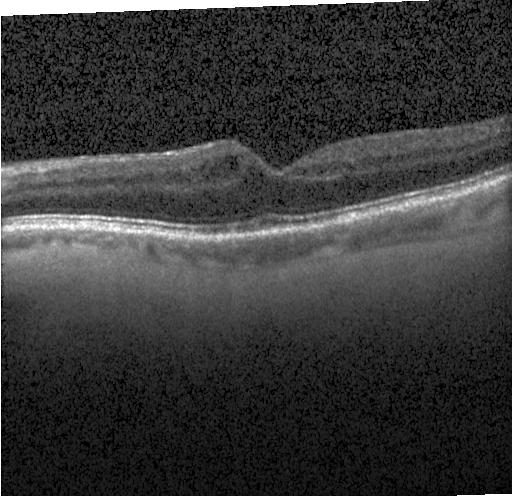

Macular scan, OCT B-scan, SD-OCT — DME.